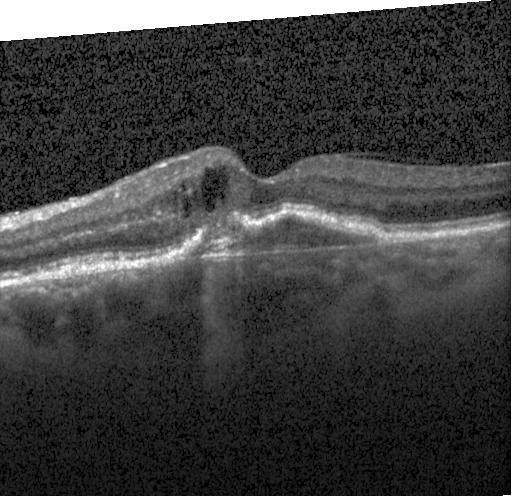

Spectral-domain OCT · macular scan · Heidelberg Spectralis OCT system · OCT line scan.
Macular OCT: a choroidal neovascular membrane.